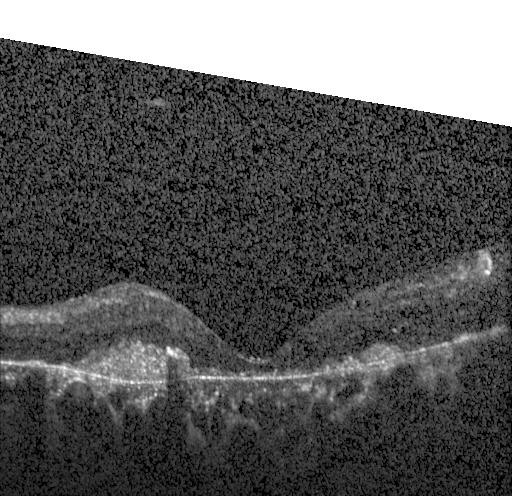
Assessment: a choroidal neovascular membrane.